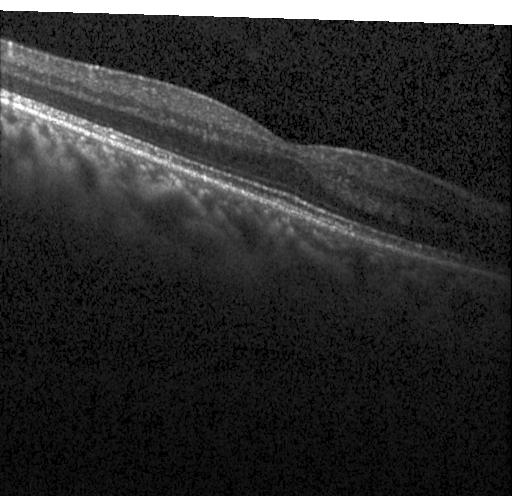 Optical coherence tomography B-scan, instrument: Heidelberg Spectralis, macular scan, spectral-domain OCT
OCT finding: no choroidal neovascularization, no diabetic macular edema, and no drusen.